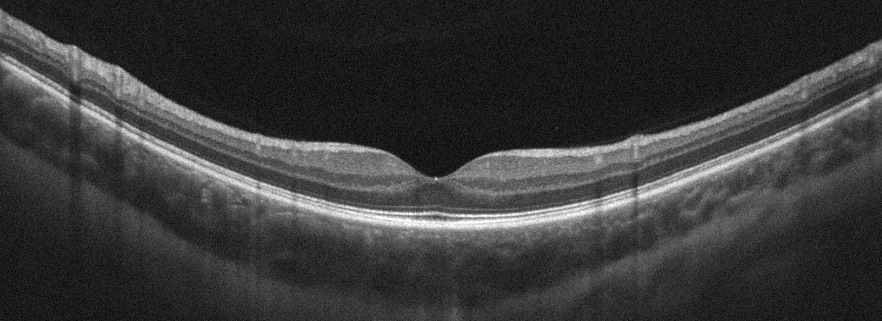 This B-scan demonstrates absence of AMD, DME, ERM, RAO, RVO, and vitreomacular interface disease.